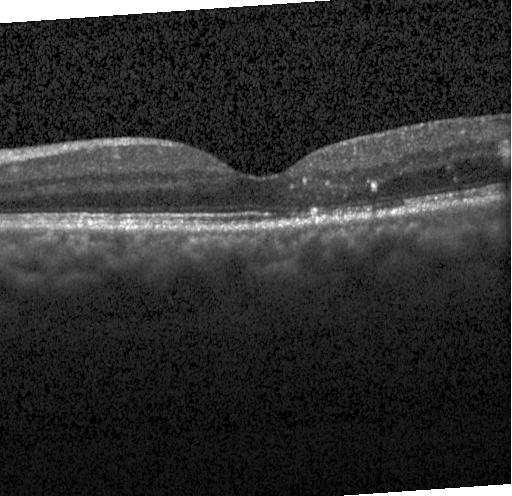
Retinal OCT cross-section. Spectral-domain OCT. Through the macula
Macular OCT: diabetic macular edema (DME).